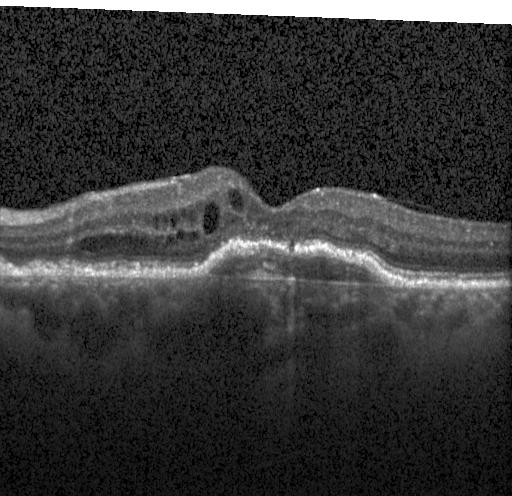 Instrument: Heidelberg Spectralis, OCT line scan.
Choroidal neovascularization (CNV).